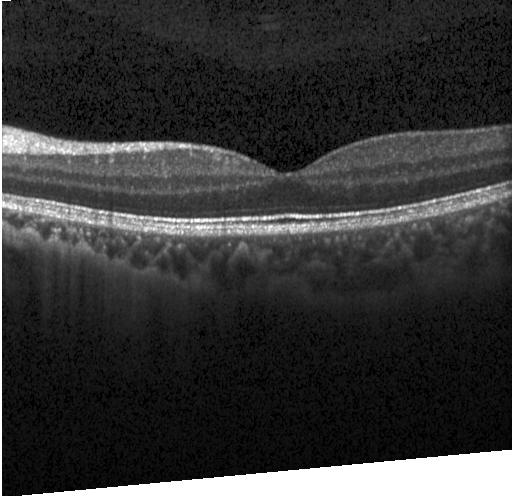
Diagnosis: no CNV, DME, or drusen.